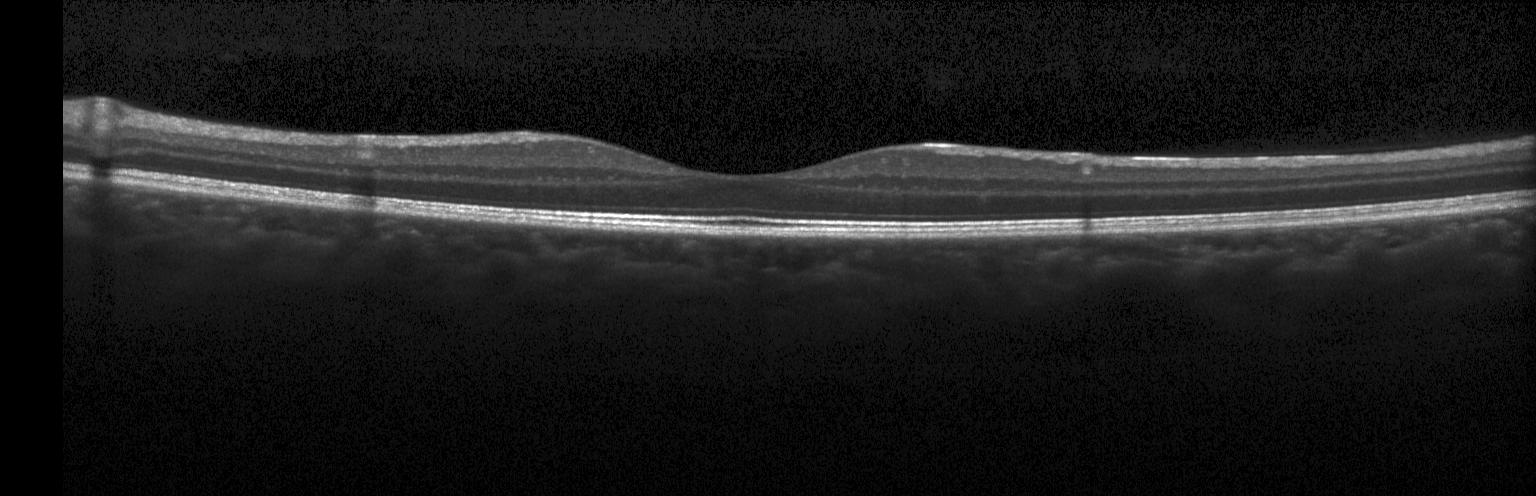
OCT line scan — Diagnosis: neither CNV, DME, nor drusen.